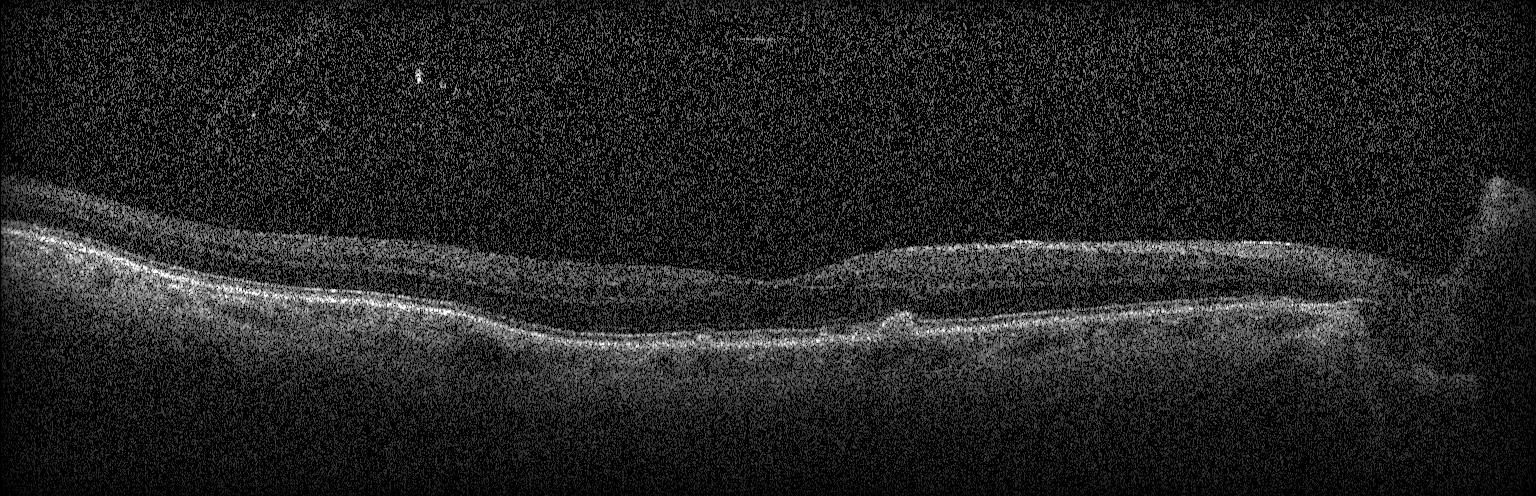

Instrument: Heidelberg Spectralis; OCT line scan
Assessment: drusen.